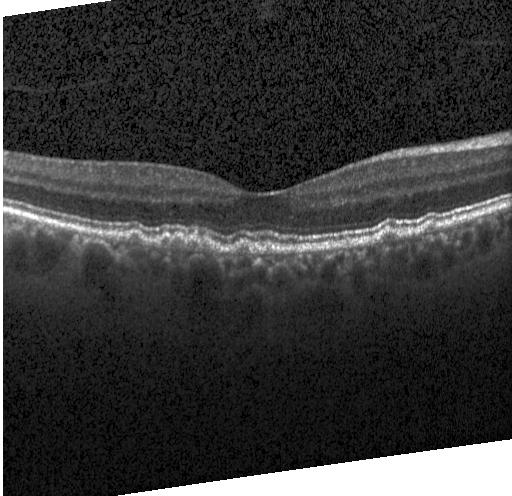

Dx: multiple drusen.